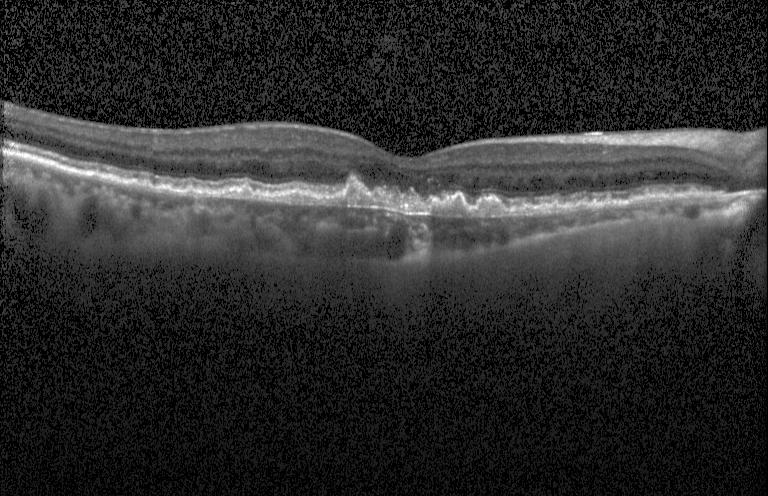
Diagnosis: choroidal neovascularization (CNV).